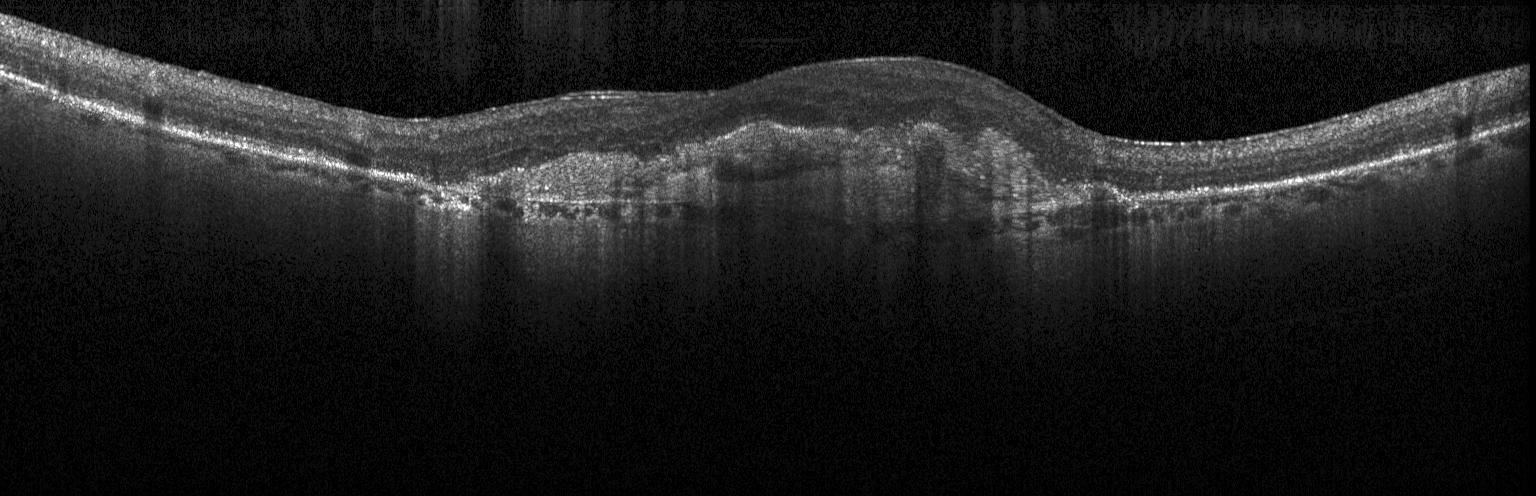 Macular OCT: a choroidal neovascular membrane.